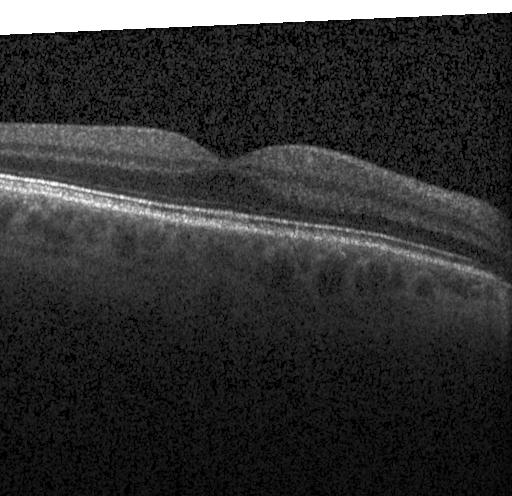 Spectral-domain OCT · Heidelberg Spectralis OCT system · centered on the fovea · retinal OCT B-scan.
The scan shows no choroidal neovascularization, diabetic macular edema, or drusen.